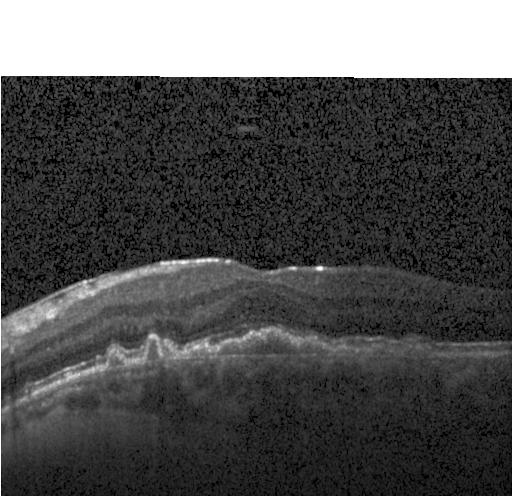

Retinal OCT cross-section — A choroidal neovascular membrane.